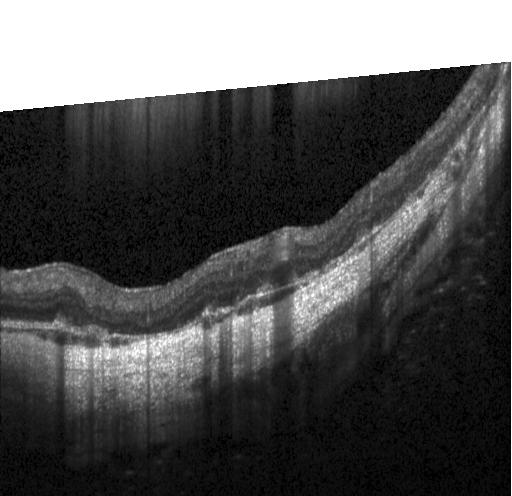 Macular scan; OCT line scan; instrument: Heidelberg Spectralis. Finding: a choroidal neovascular membrane.